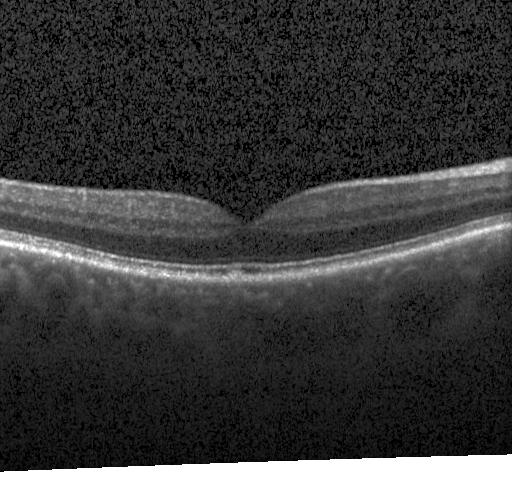

Macular OCT: no CNV, DME, or drusen.